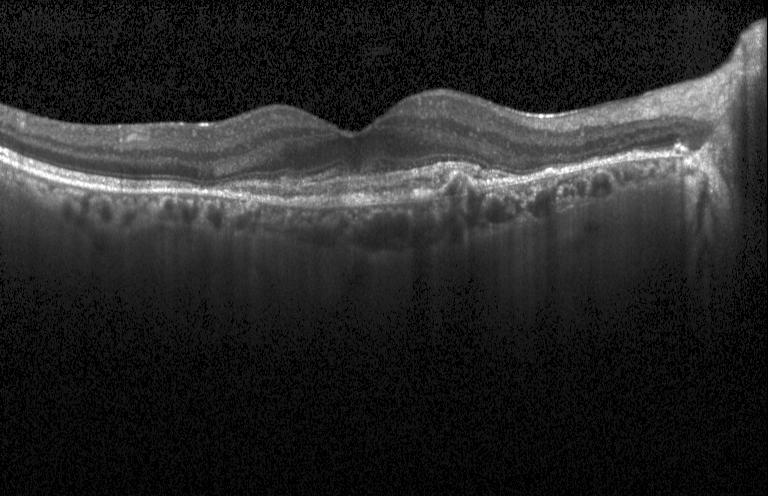
Optical coherence tomography B-scan. Through the macula. Spectral-domain OCT — Finding: choroidal neovascularization (CNV).